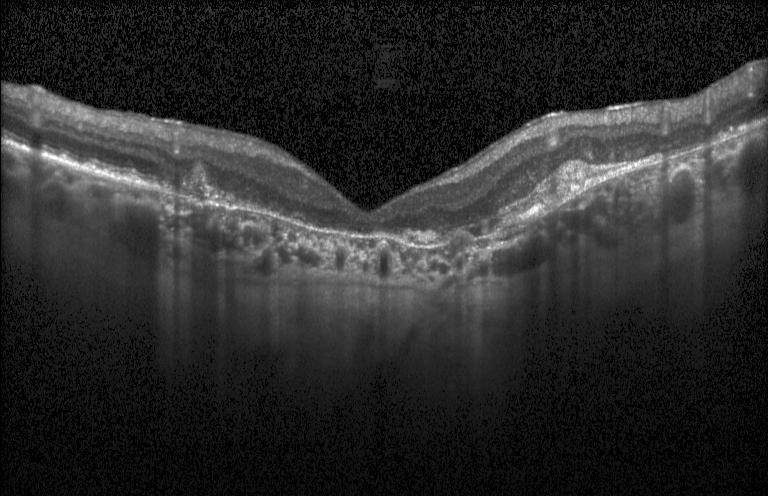 Finding: a choroidal neovascular membrane.